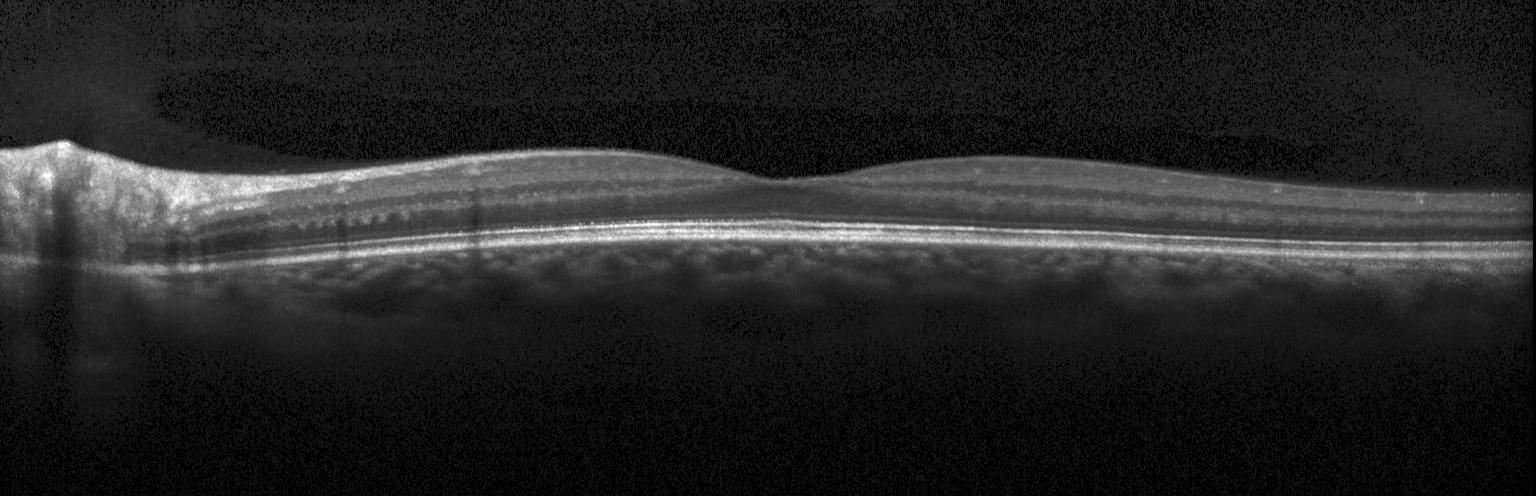
Instrument: Heidelberg Spectralis; OCT line scan; through the macula; spectral-domain OCT — Dx: no CNV, no DME, and no drusen.